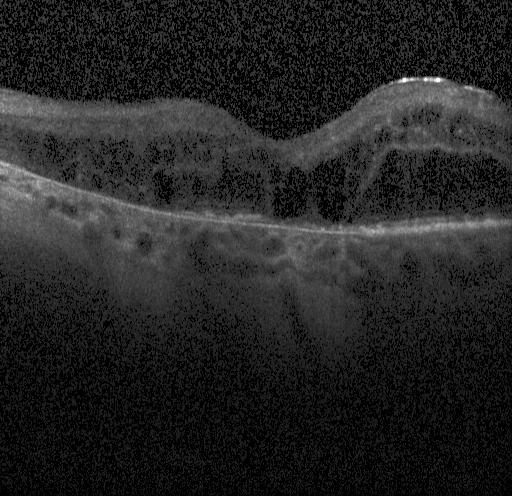

Diagnosis: CNV.